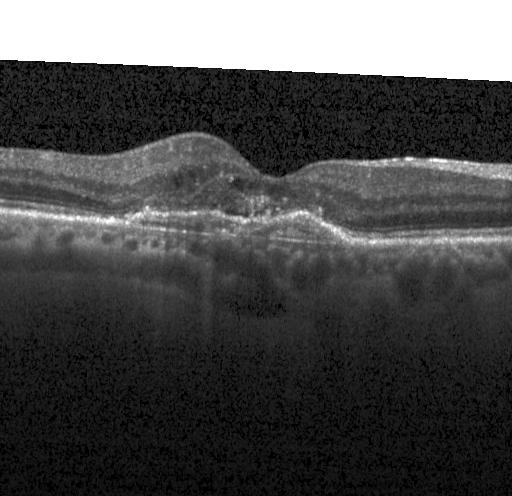

Macular OCT: a choroidal neovascular membrane.